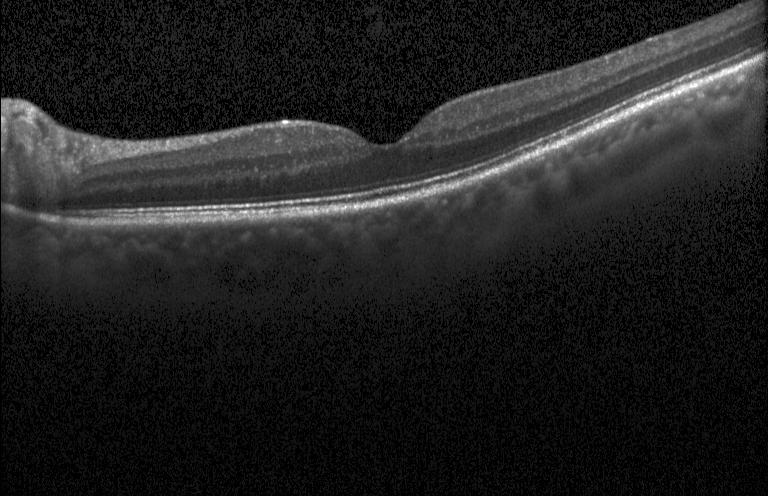

Instrument: Heidelberg Spectralis · optical coherence tomography scan · centered on the fovea.
Assessment: neither CNV, DME, nor drusen.